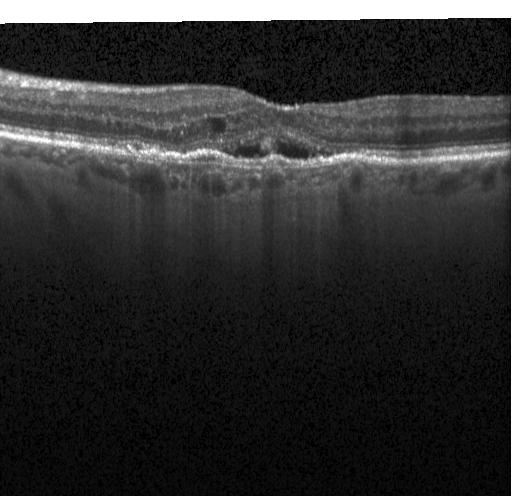
This B-scan demonstrates choroidal neovascularization (CNV).